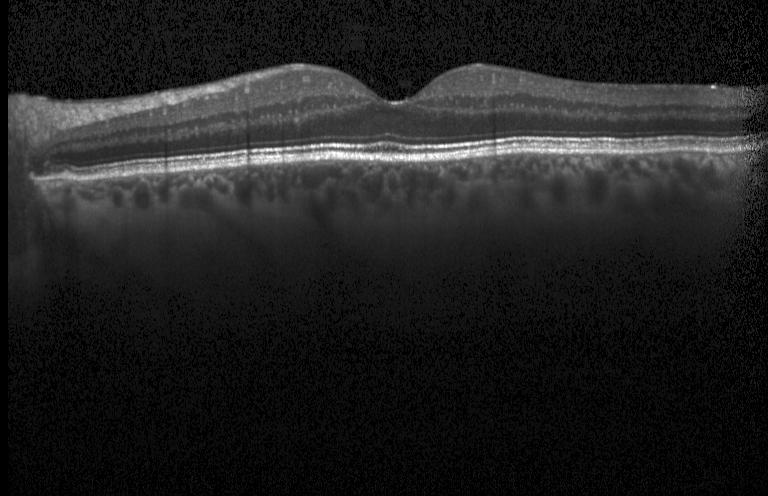

OCT B-scan showing no CNV, no DME, and no drusen.